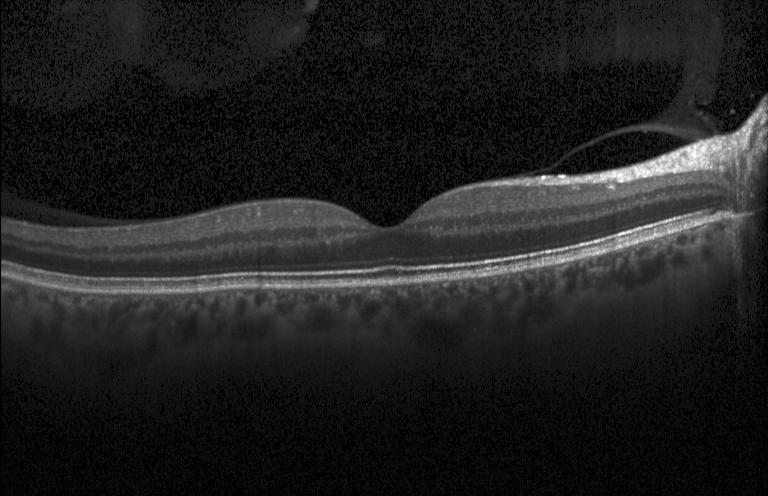

OCT scan showing no choroidal neovascularization, no diabetic macular edema, and no drusen.